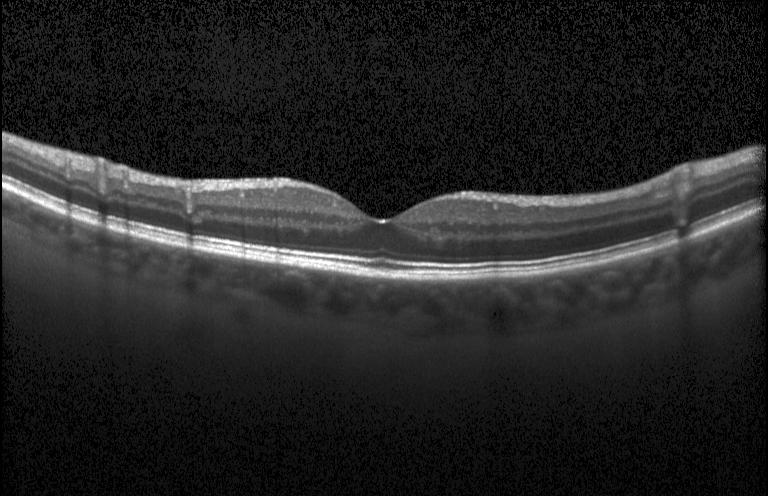 Retinal OCT B-scan.
This B-scan demonstrates no choroidal neovascularization, no diabetic macular edema, and no drusen.